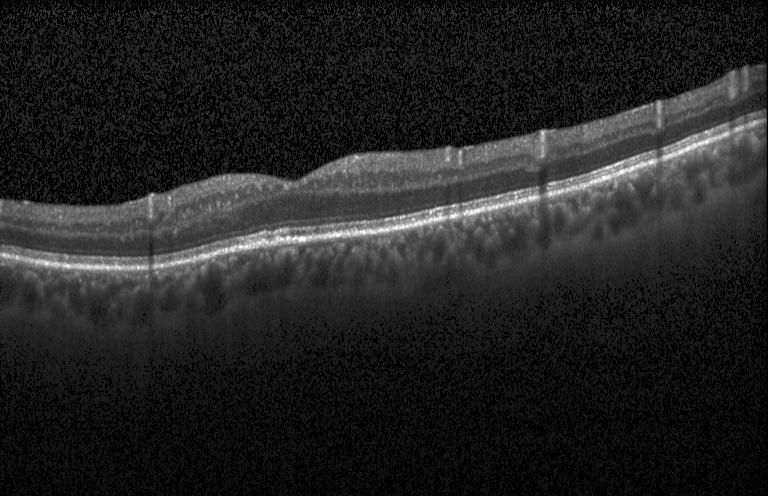

Dx: neither CNV, DME, nor drusen.